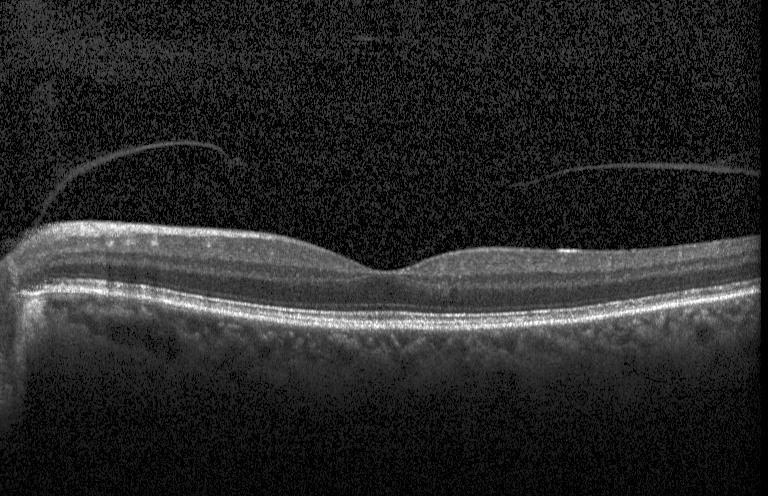
Spectral-domain optical coherence tomography · optical coherence tomography B-scan
Impression: no choroidal neovascularization, diabetic macular edema, or drusen.